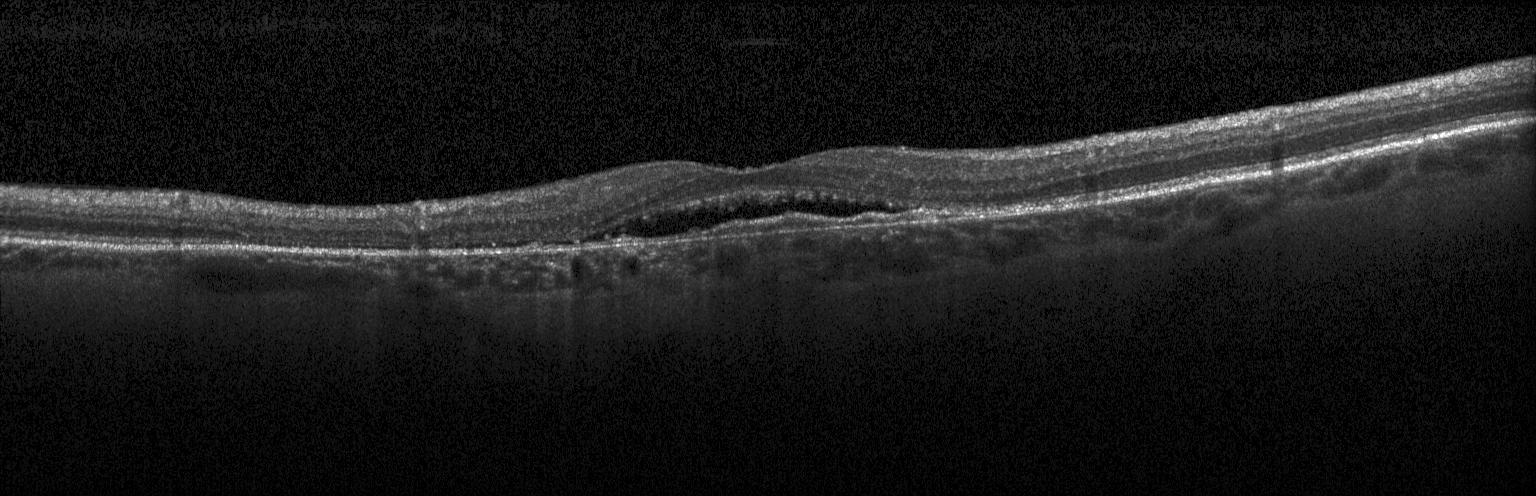

Heidelberg Spectralis OCT system · OCT B-scan.
Impression: choroidal neovascularization.